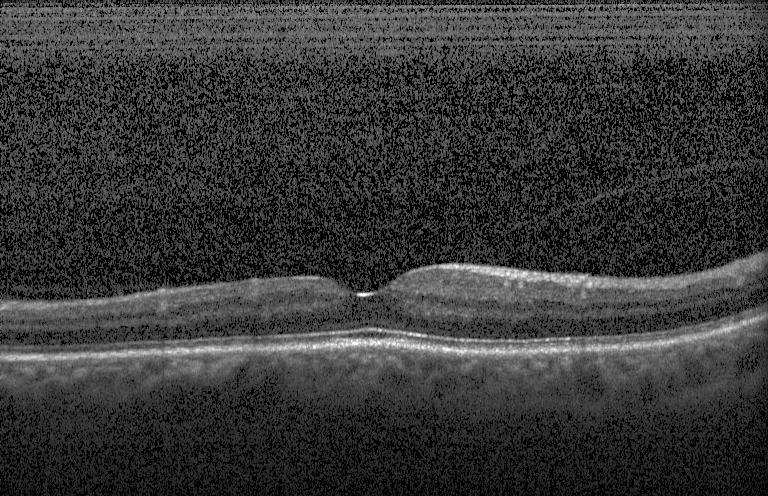 Retinal OCT B-scan — Diagnosis: no CNV, DME, or drusen.